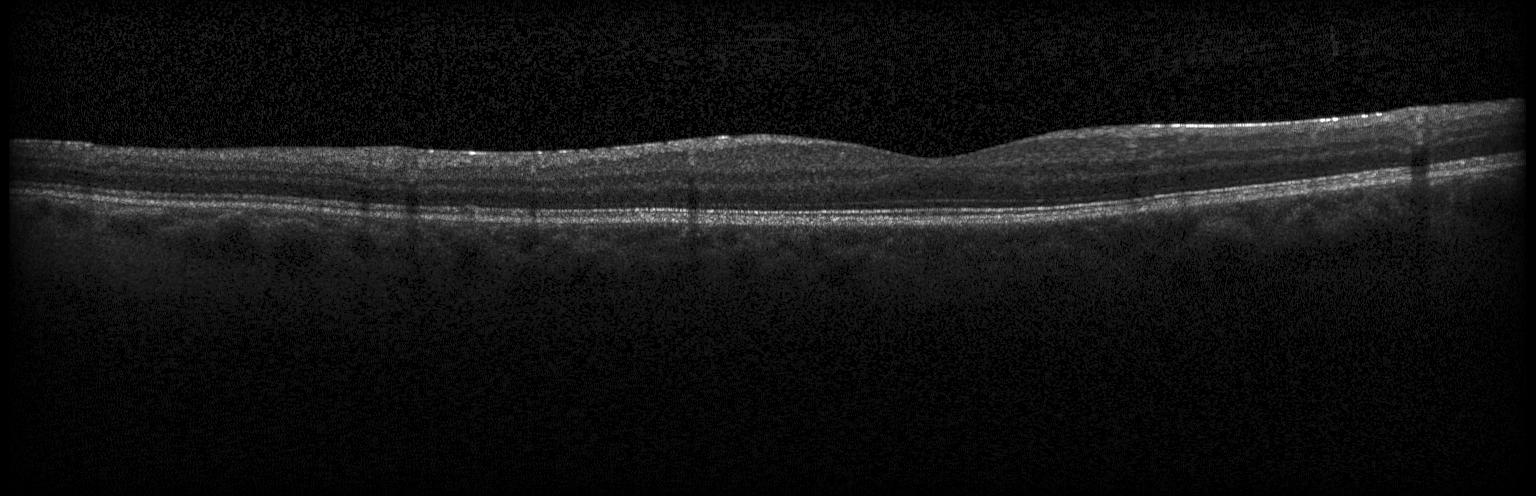
No choroidal neovascularization, no diabetic macular edema, and no drusen.